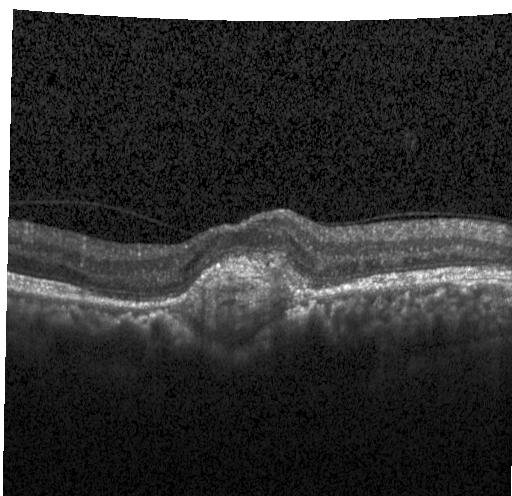
Centered on the fovea · OCT line scan · Heidelberg Spectralis OCT system · spectral-domain OCT
Macular OCT: choroidal neovascularization (CNV).